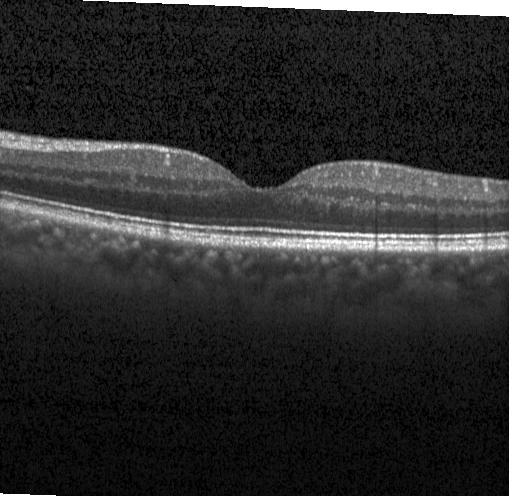

Retinal OCT cross-section — Finding: no CNV, DME, or drusen.